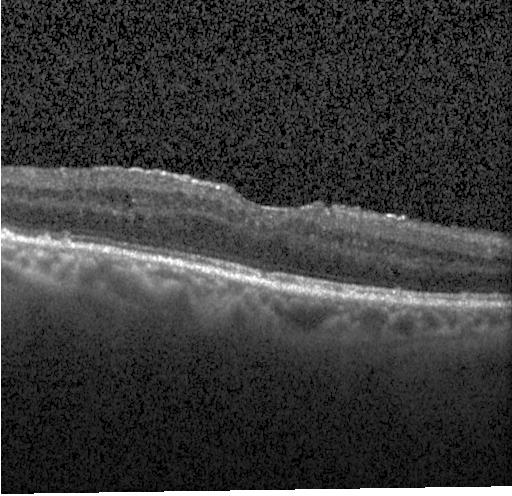

Macular OCT demonstrating diabetic macular edema.